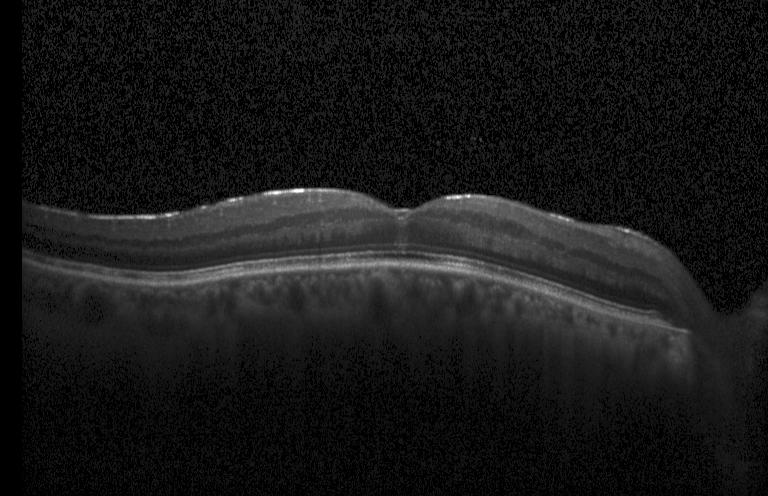
Retinal OCT B-scan, Heidelberg Spectralis, macular scan, spectral-domain optical coherence tomography — Impression: no evidence of CNV, DME, or drusen.